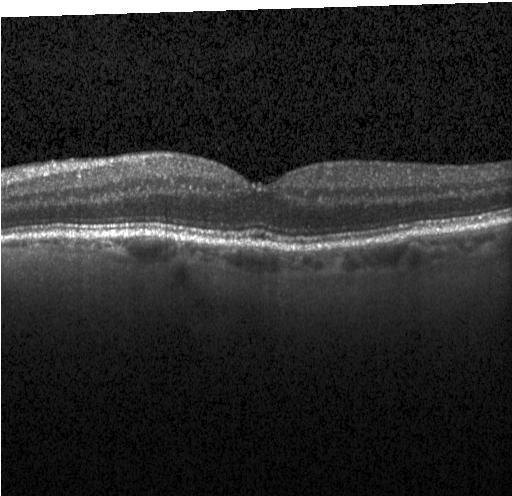
Through the macula; optical coherence tomography scan. Finding: neither choroidal neovascularization, diabetic macular edema, nor drusen.